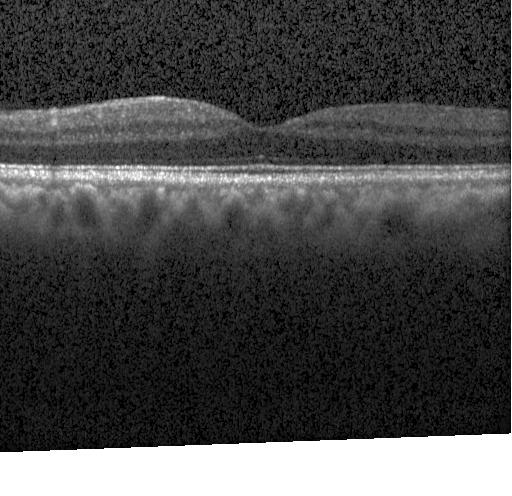 Retinal OCT cross-section; spectral-domain optical coherence tomography
Diagnosis: no evidence of CNV, DME, or drusen.